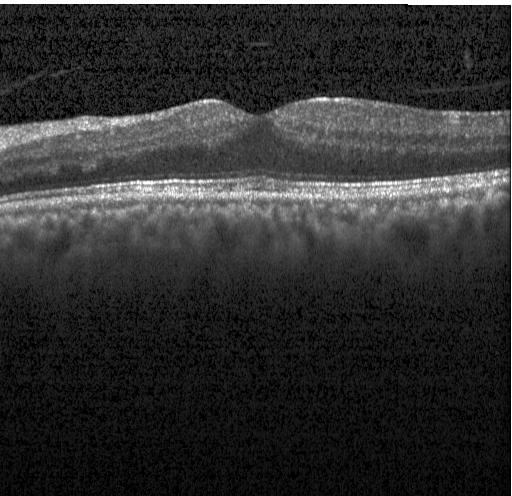
Fovea-centered. Retinal OCT B-scan. Heidelberg Spectralis OCT system
Finding: no evidence of choroidal neovascularization, diabetic macular edema, or drusen.